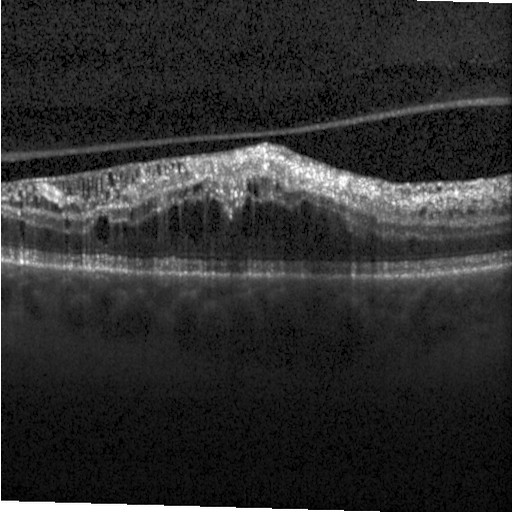

Impression: diabetic macular edema.